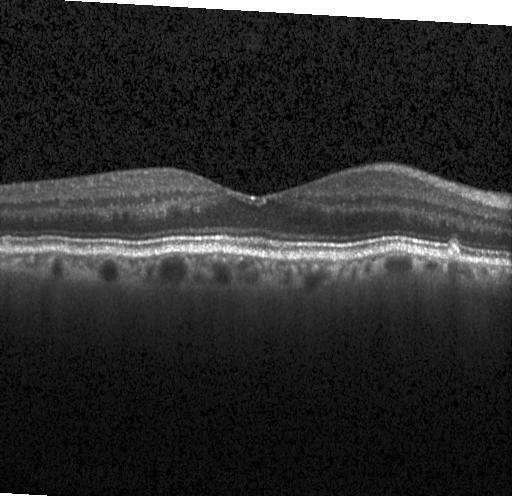 Retinal OCT cross-section. Diagnosis: no CNV, DME, or drusen.